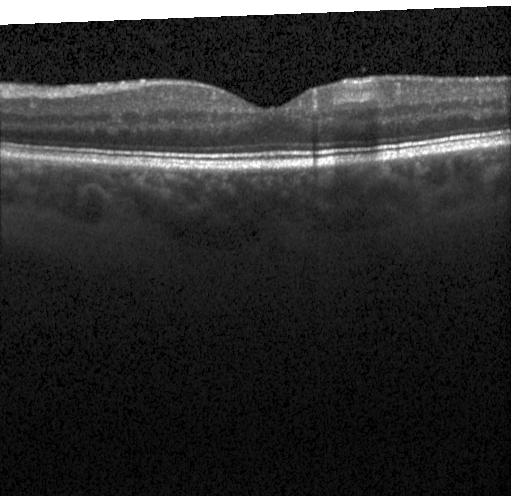

Retinal OCT B-scan; instrument: Heidelberg Spectralis
No choroidal neovascularization, no diabetic macular edema, and no drusen.